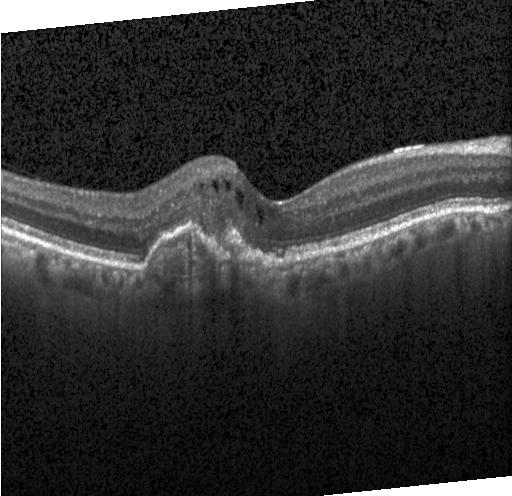 A choroidal neovascular membrane.